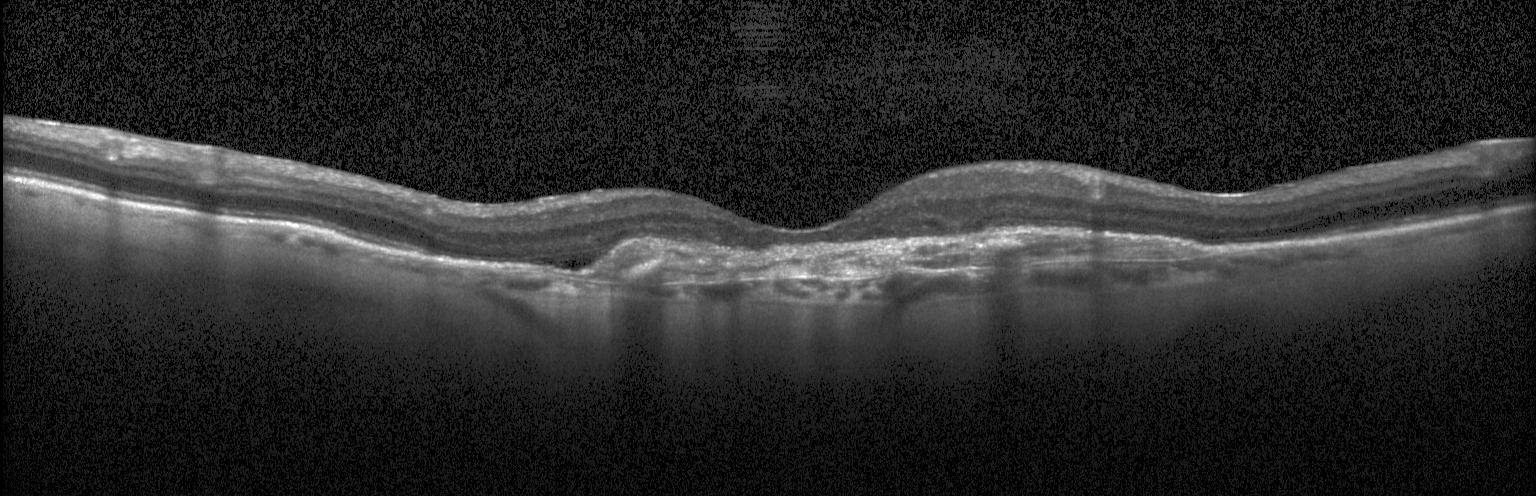 Optical coherence tomography B-scan
Impression: choroidal neovascularization (CNV).